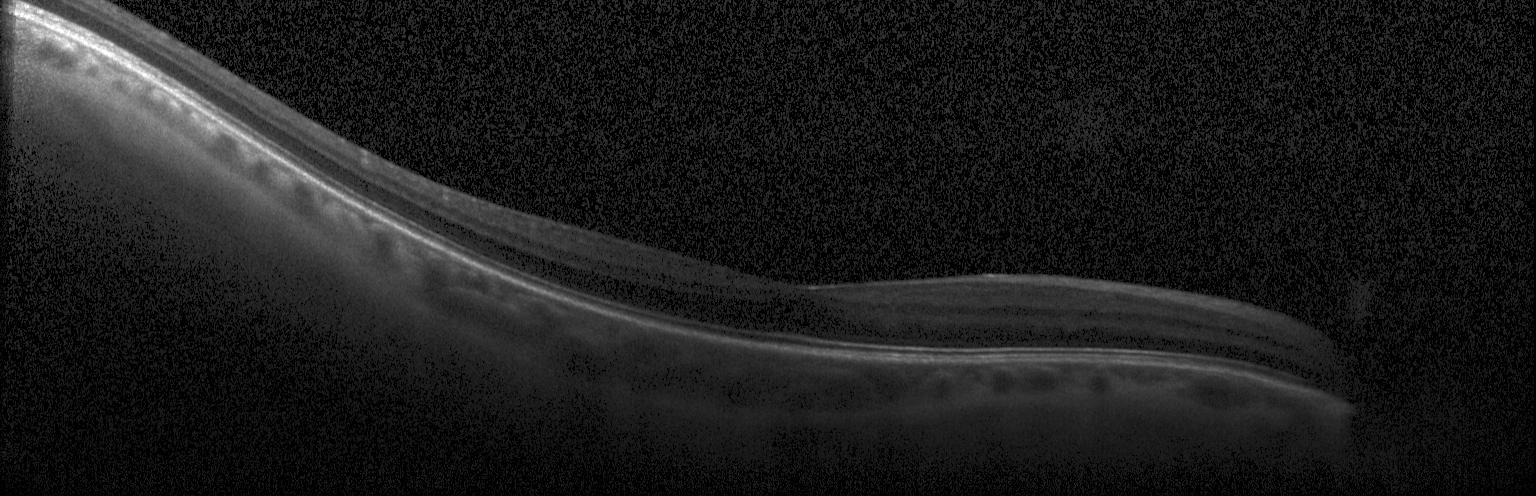
Spectral-domain OCT. OCT B-scan.
Assessment: no evidence of CNV, DME, or drusen.